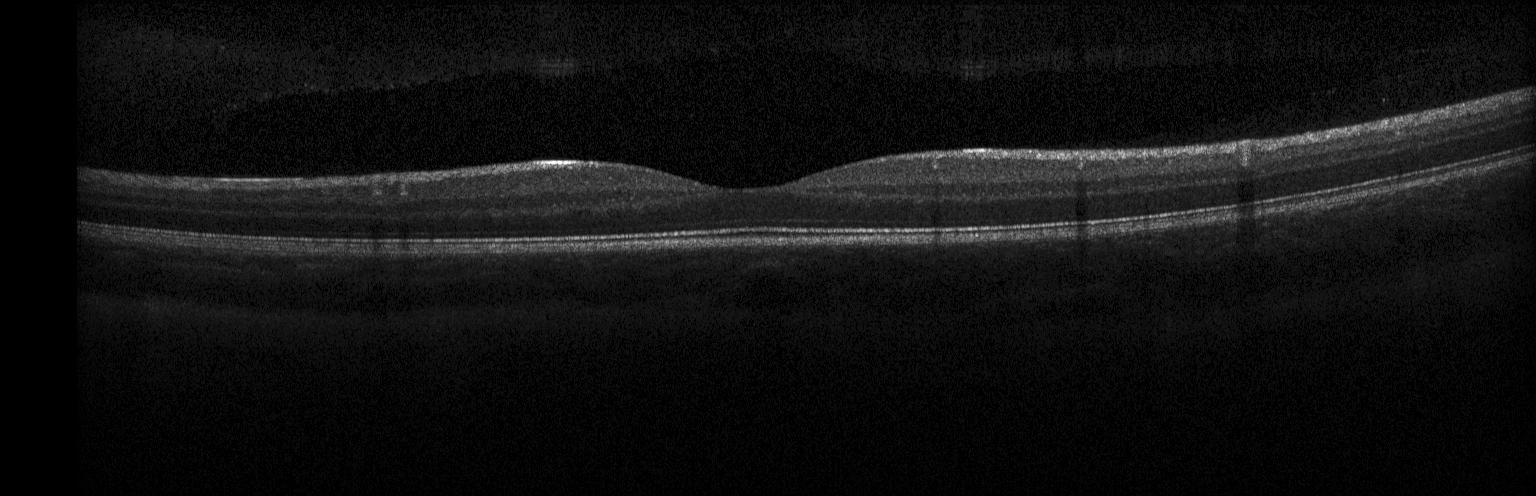
OCT finding: no evidence of choroidal neovascularization, diabetic macular edema, or drusen.